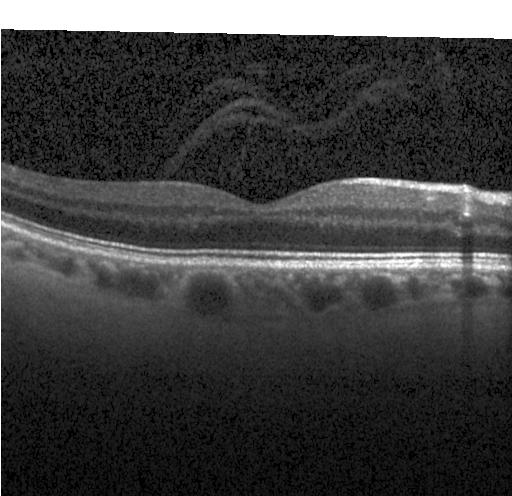
OCT B-scan
Macular OCT: no CNV, no DME, and no drusen.